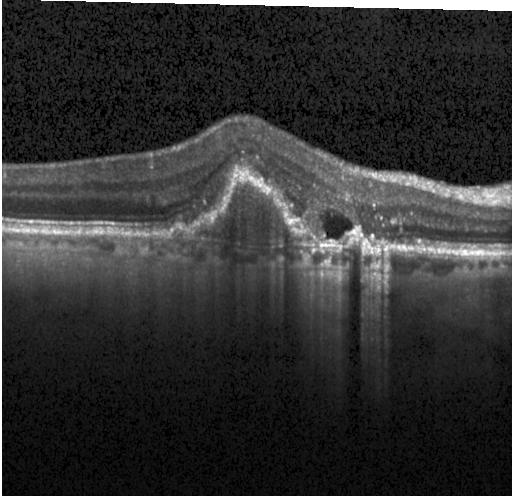

OCT B-scan — Finding: choroidal neovascularization (CNV).